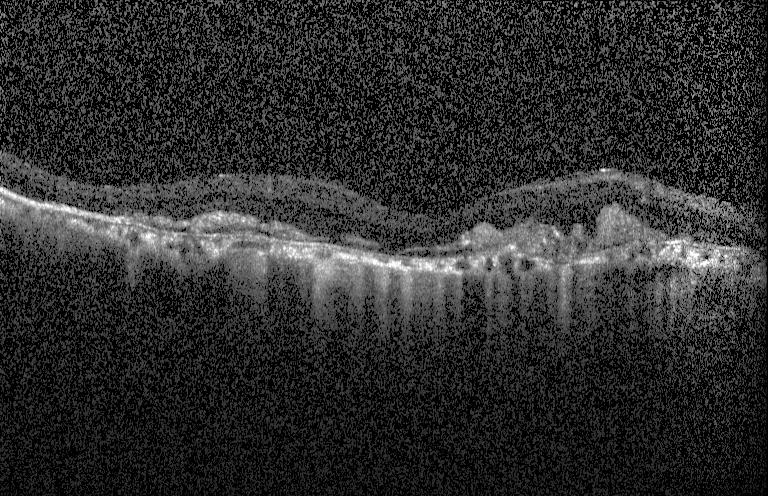 Acquired on a Heidelberg Spectralis; optical coherence tomography scan; through the macula; SD-OCT. Dx: choroidal neovascularization.